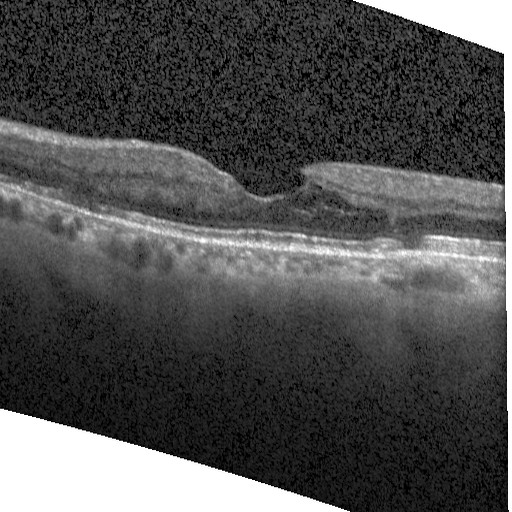 Finding: DME.